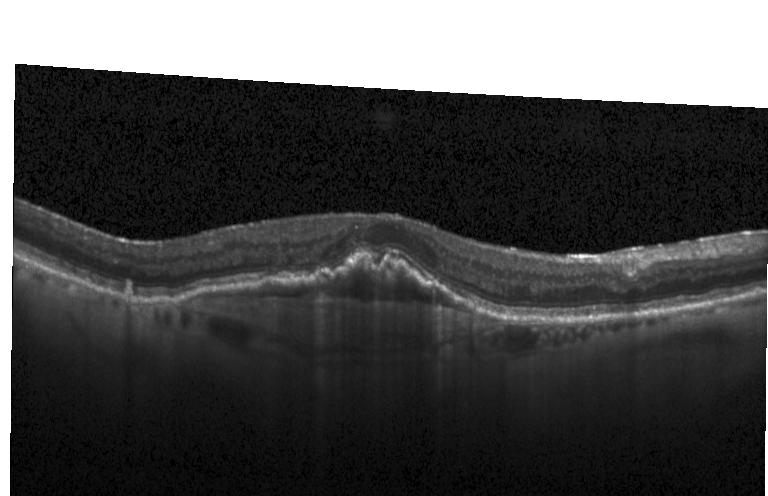 Diagnosis: a choroidal neovascular membrane.